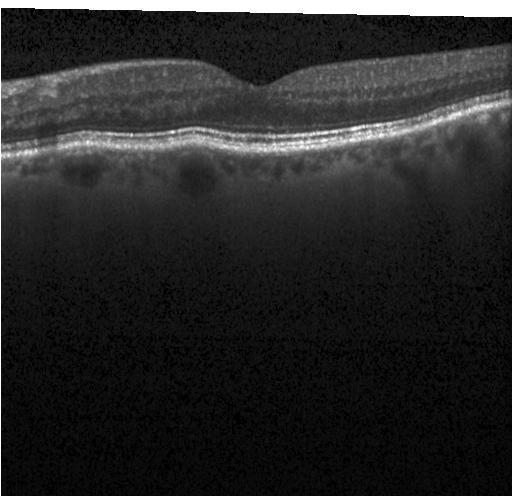

Optical coherence tomography scan. Spectral-domain optical coherence tomography. Impression: no evidence of choroidal neovascularization, diabetic macular edema, or drusen.